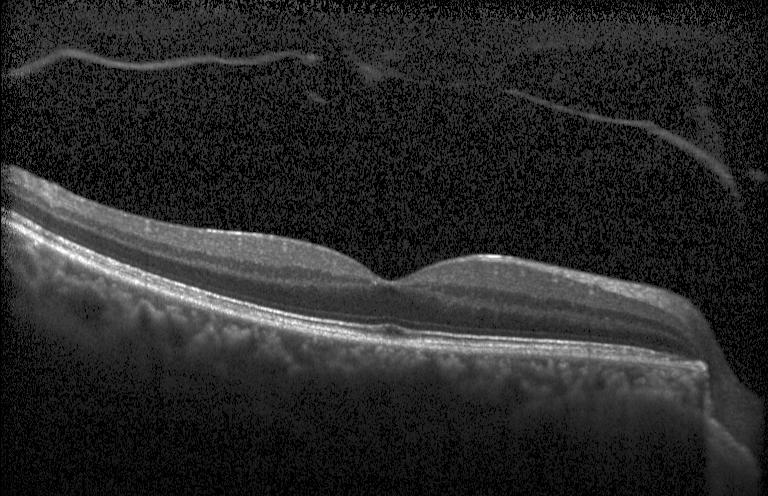
Dx: no CNV, DME, or drusen.